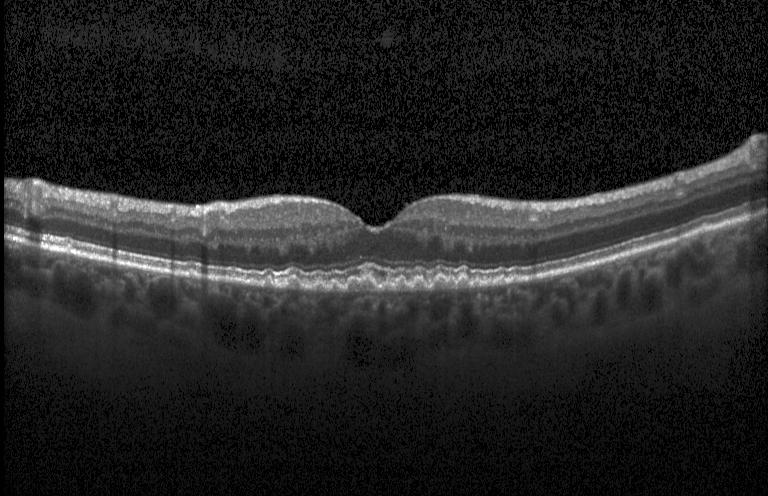 Retinal OCT cross-section, acquired on a Heidelberg Spectralis.
Diagnosis: sub-RPE drusenoid deposits.